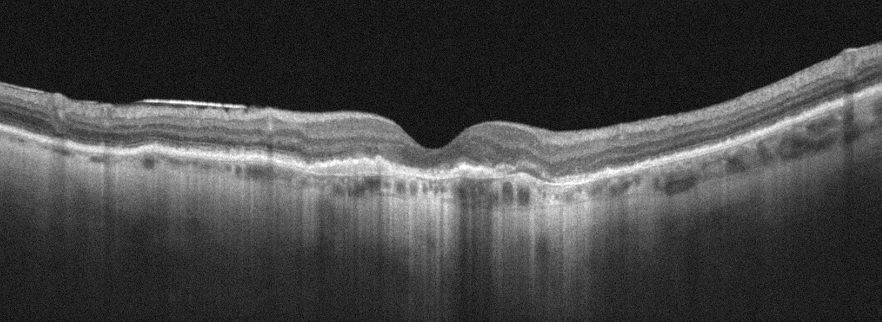 Through the macula · oculus sinister · retinal OCT cross-section — Dx: age-related macular degeneration.